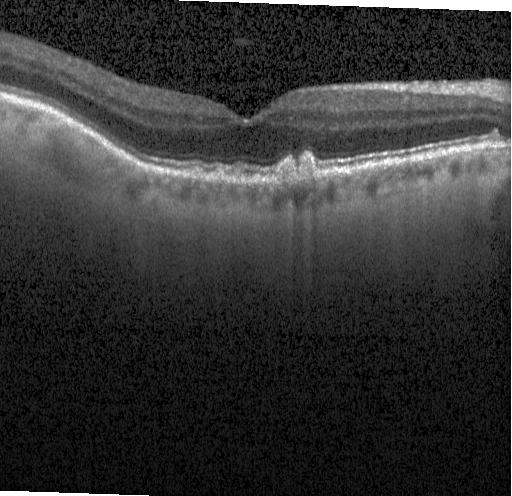 Assessment: multiple drusen.